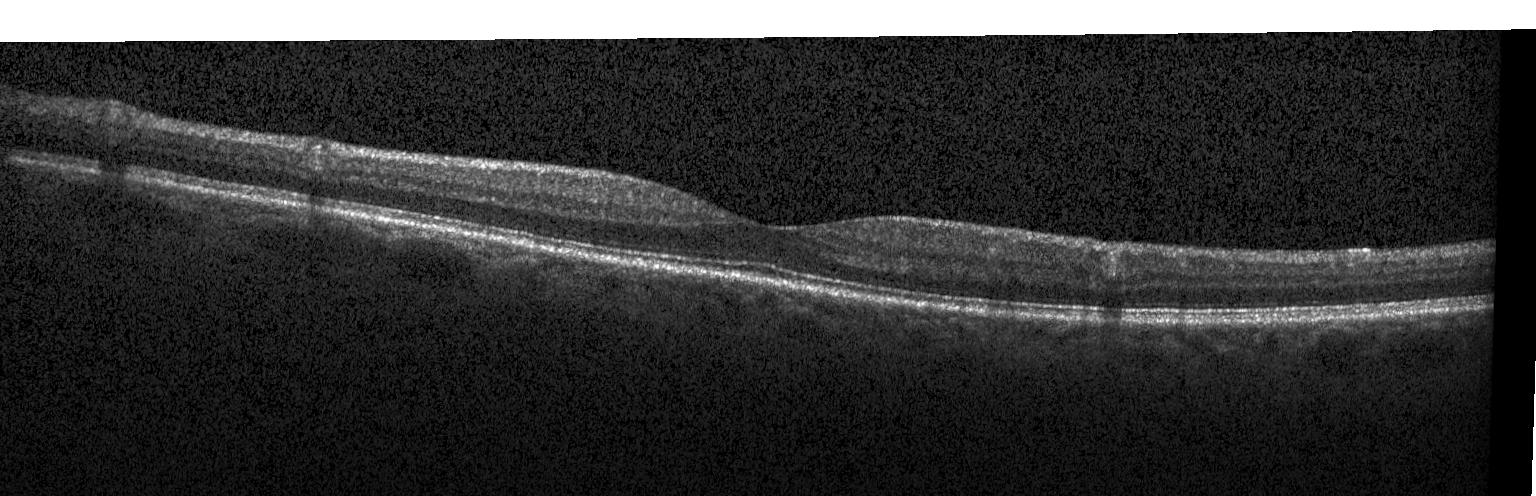 Optical coherence tomography scan · horizontal scan through the fovea.
Assessment: no evidence of CNV, DME, or drusen.